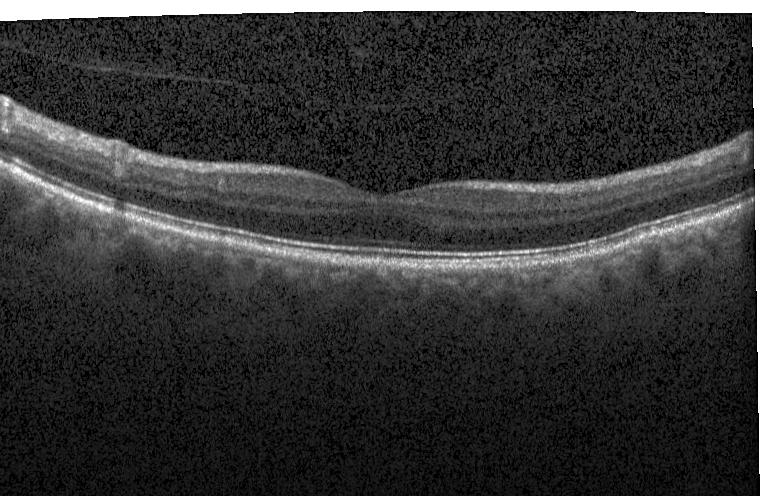 OCT line scan, Heidelberg Spectralis OCT system, SD-OCT, centered on the fovea.
Macular OCT: no evidence of choroidal neovascularization, diabetic macular edema, or drusen.